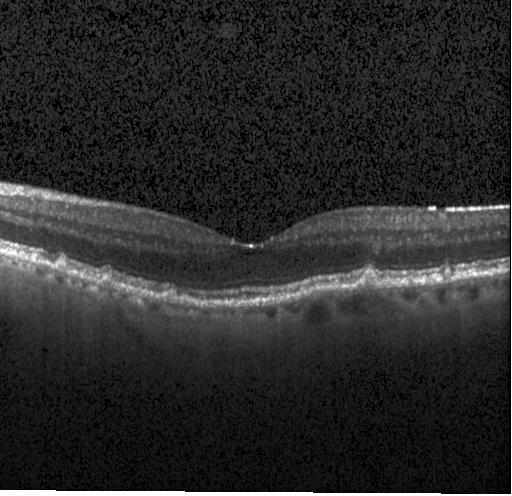

Impression: sub-RPE drusenoid deposits.